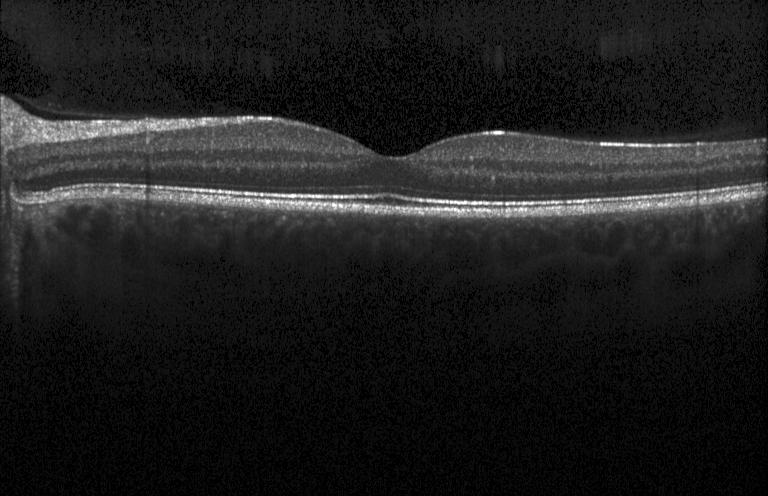
No evidence of CNV, DME, or drusen.